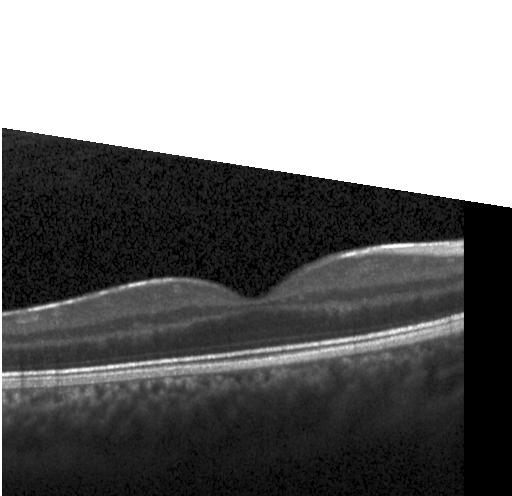
OCT scan showing no CNV, no DME, and no drusen.